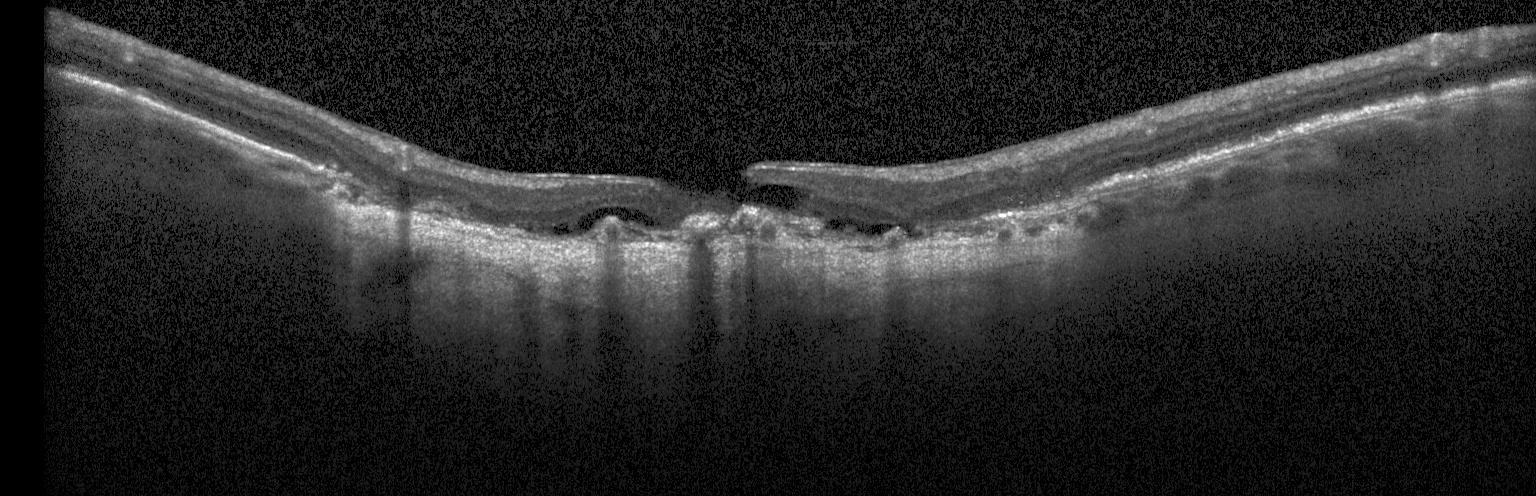 Retinal OCT B-scan
Assessment: choroidal neovascularization.